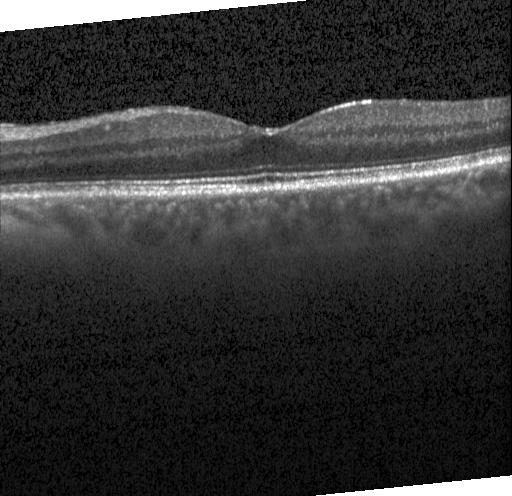

Impression: no choroidal neovascularization, no diabetic macular edema, and no drusen.